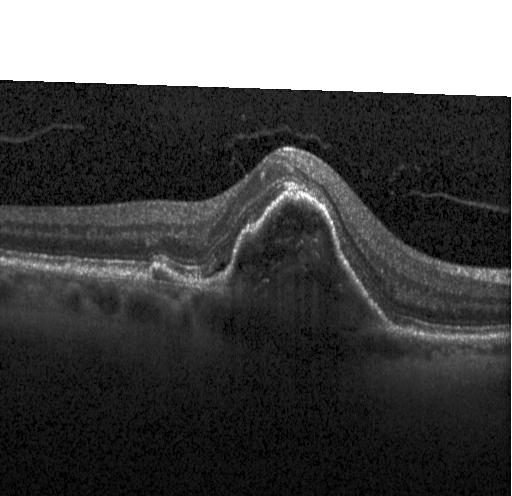 SD-OCT; centered on the fovea; OCT B-scan.
OCT finding: choroidal neovascularization.